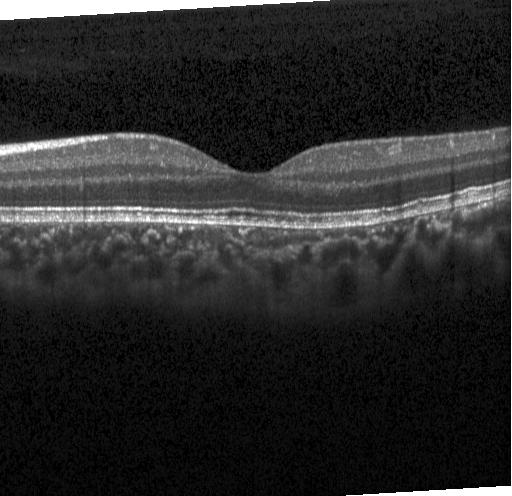
Optical coherence tomography B-scan — Diagnosis: no choroidal neovascularization, diabetic macular edema, or drusen.